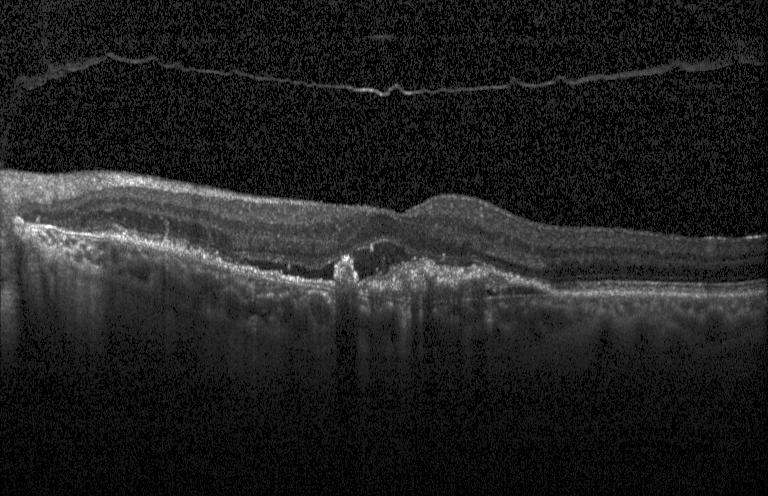

The scan shows choroidal neovascularization.